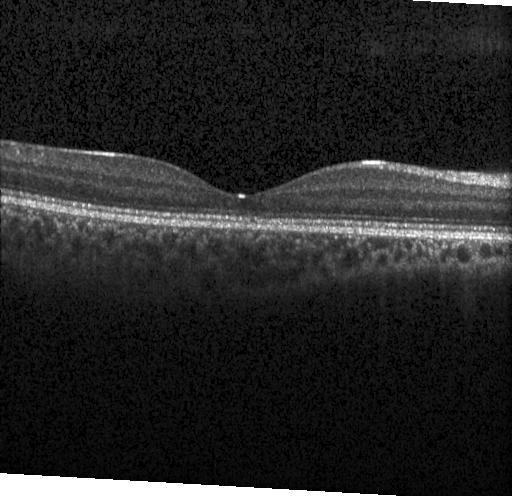

Macular OCT demonstrating neither CNV, DME, nor drusen.